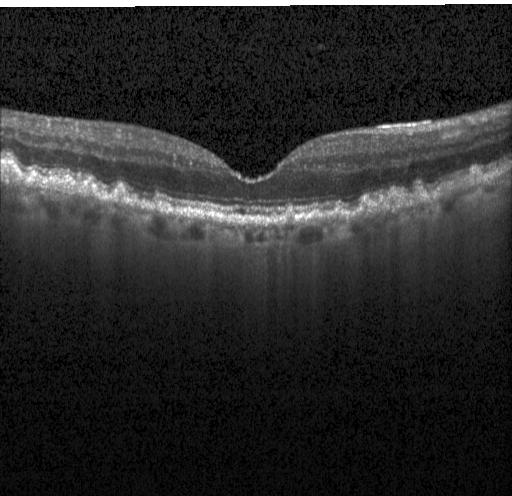
Through the macula · retinal OCT cross-section. Diagnosis: multiple drusen.